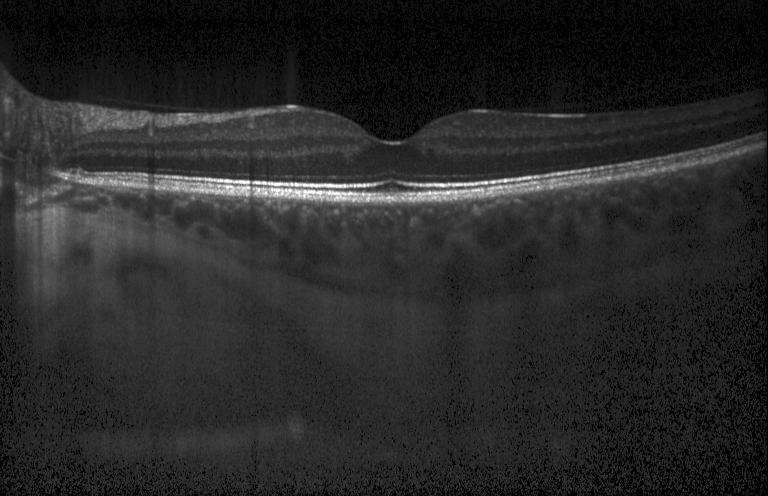
Retinal OCT cross-section; SD-OCT — Finding: no CNV, DME, or drusen.